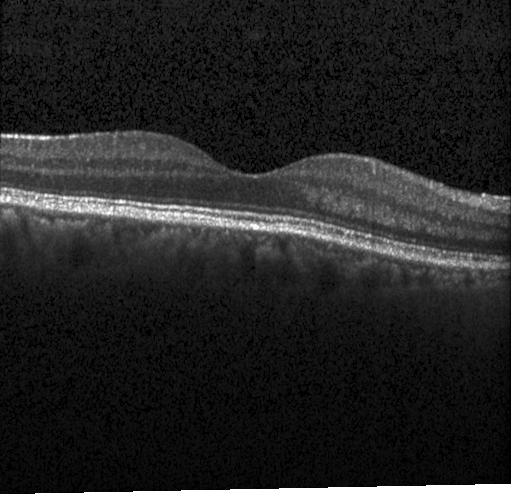 Retinal OCT B-scan — Diagnosis: no choroidal neovascularization, no diabetic macular edema, and no drusen.